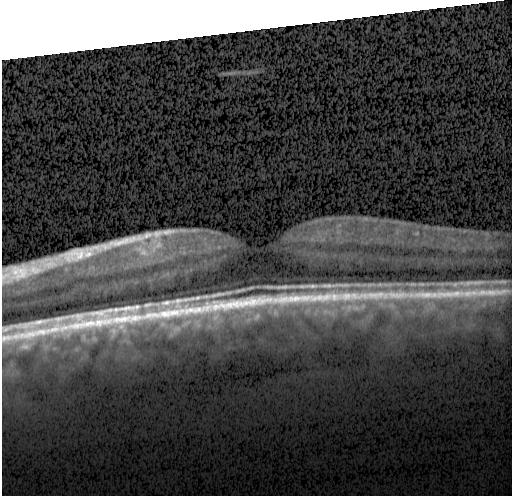 OCT B-scan
Finding: no choroidal neovascularization, diabetic macular edema, or drusen.